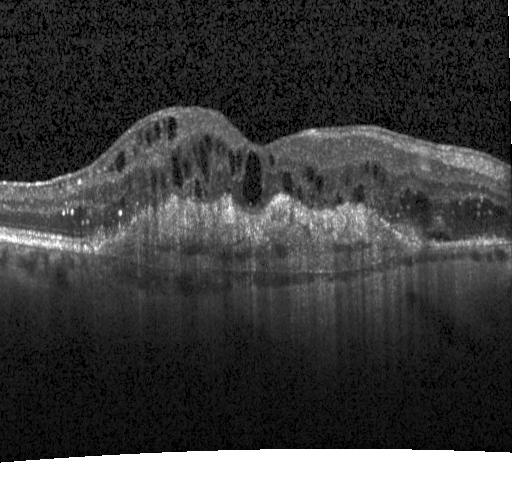

Optical coherence tomography scan. Spectral-domain OCT
Finding: choroidal neovascularization.